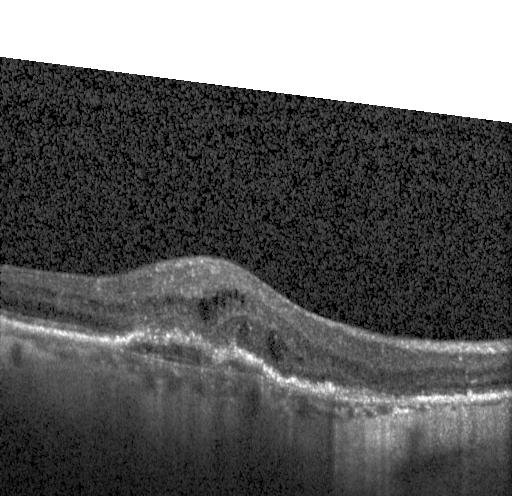 Spectral-domain optical coherence tomography · optical coherence tomography scan
Diagnosis: a choroidal neovascular membrane.